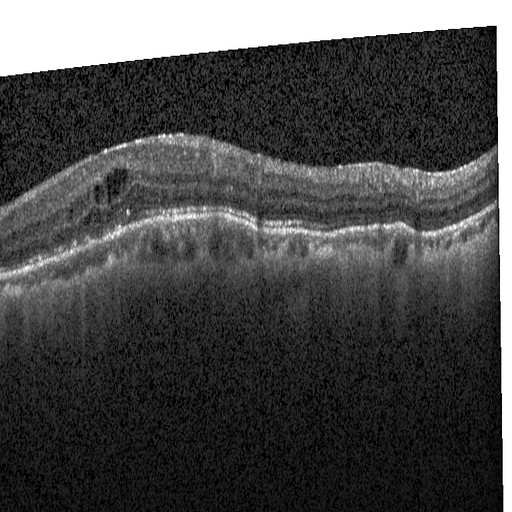
Through the macula, acquired on a Heidelberg Spectralis, SD-OCT, retinal OCT B-scan.
Impression: diabetic macular edema.